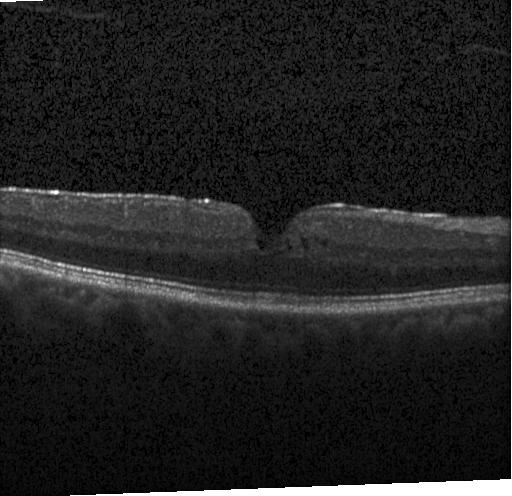 Assessment: DME.